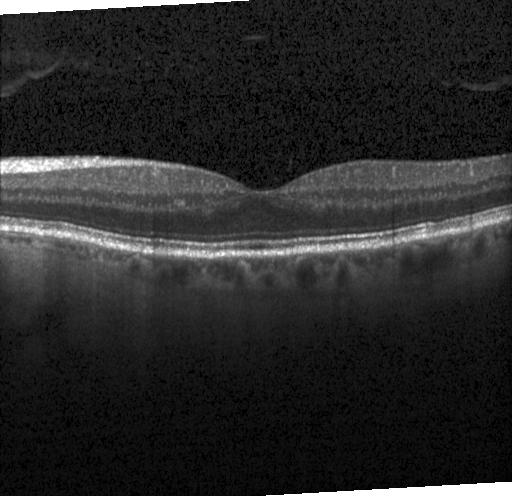

OCT B-scan showing no CNV, DME, or drusen.